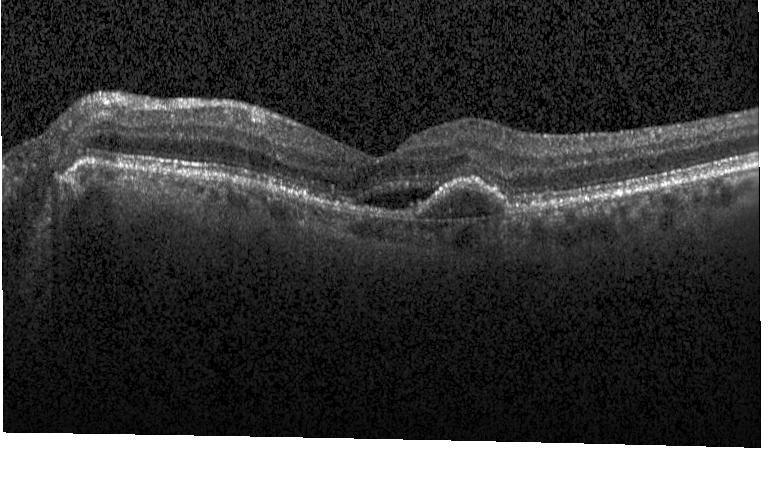 Optical coherence tomography scan. Diagnosis: choroidal neovascularization.